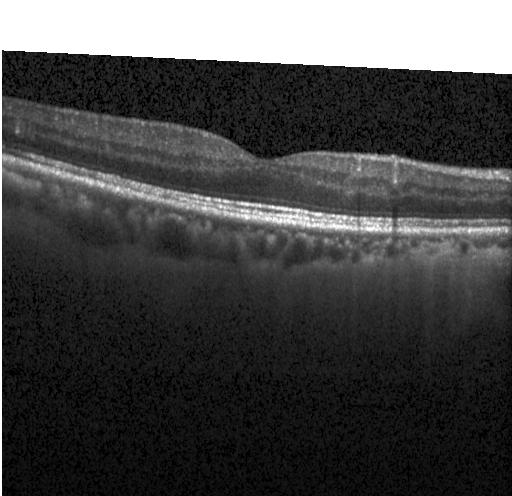
Optical coherence tomography B-scan. Centered on the fovea.
Diagnosis: no evidence of CNV, DME, or drusen.